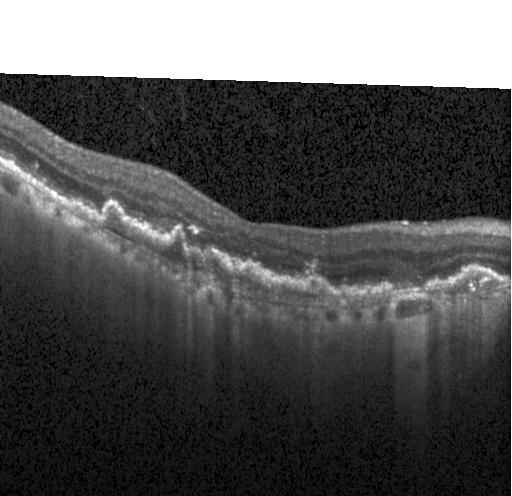 Instrument: Heidelberg Spectralis · optical coherence tomography B-scan · SD-OCT.
A choroidal neovascular membrane.